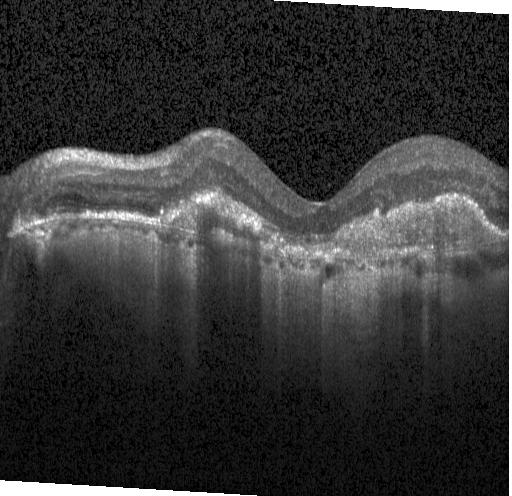
CNV.